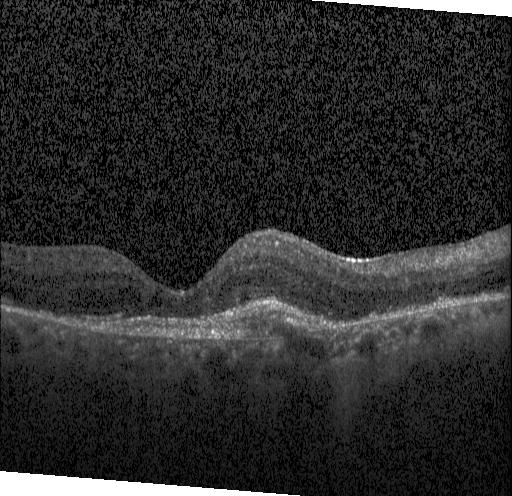
SD-OCT. Fovea-centered. Acquired on a Heidelberg Spectralis. Retinal OCT B-scan. The scan shows choroidal neovascularization.